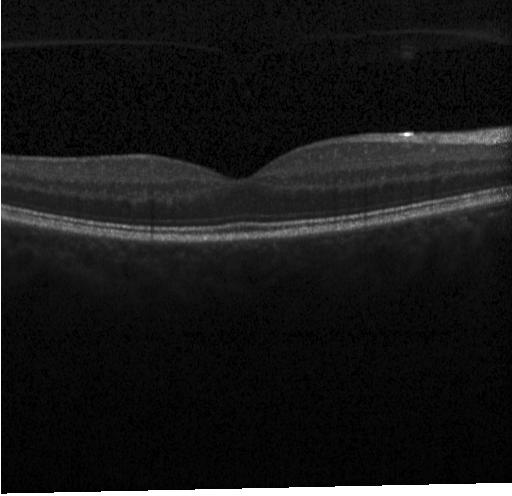
Optical coherence tomography scan · horizontal scan through the fovea
The scan shows no choroidal neovascularization, no diabetic macular edema, and no drusen.